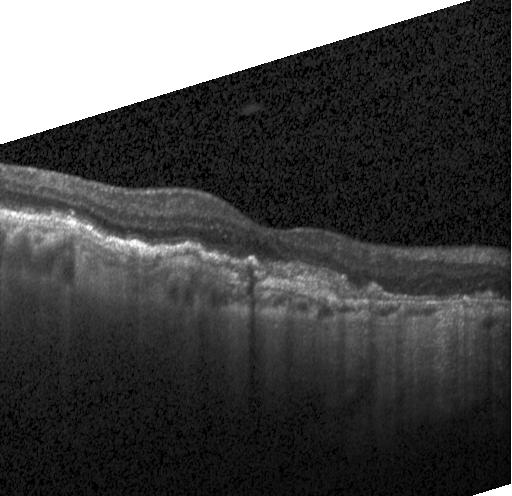

Spectral-domain OCT B-scan: choroidal neovascularization.